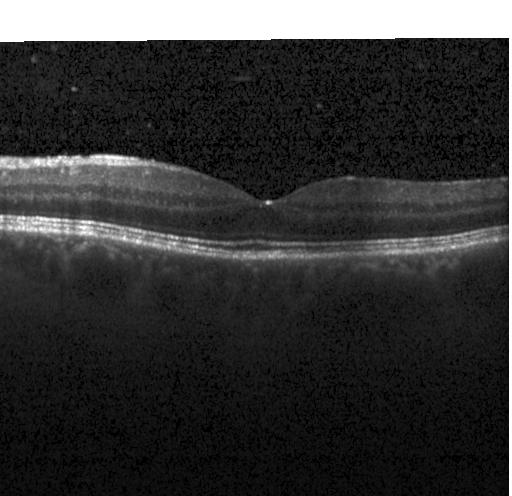 Impression: neither choroidal neovascularization, diabetic macular edema, nor drusen.